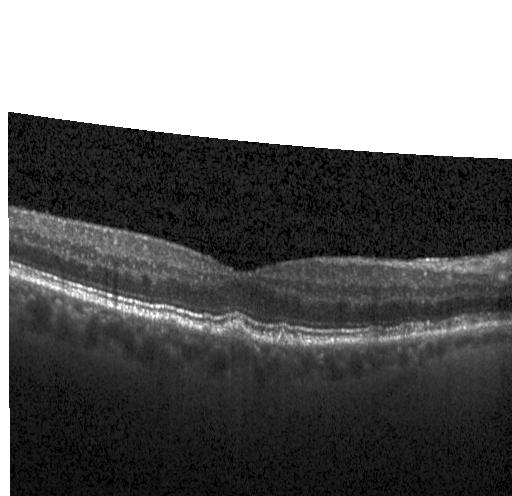
Drusen.